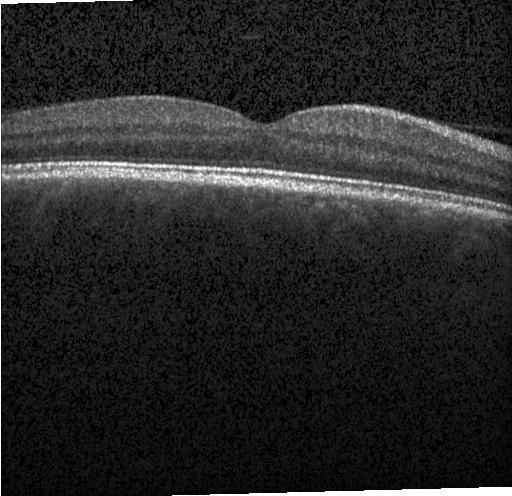
OCT line scan, SD-OCT, acquired on a Heidelberg Spectralis, centered on the fovea
Assessment: no choroidal neovascularization, no diabetic macular edema, and no drusen.